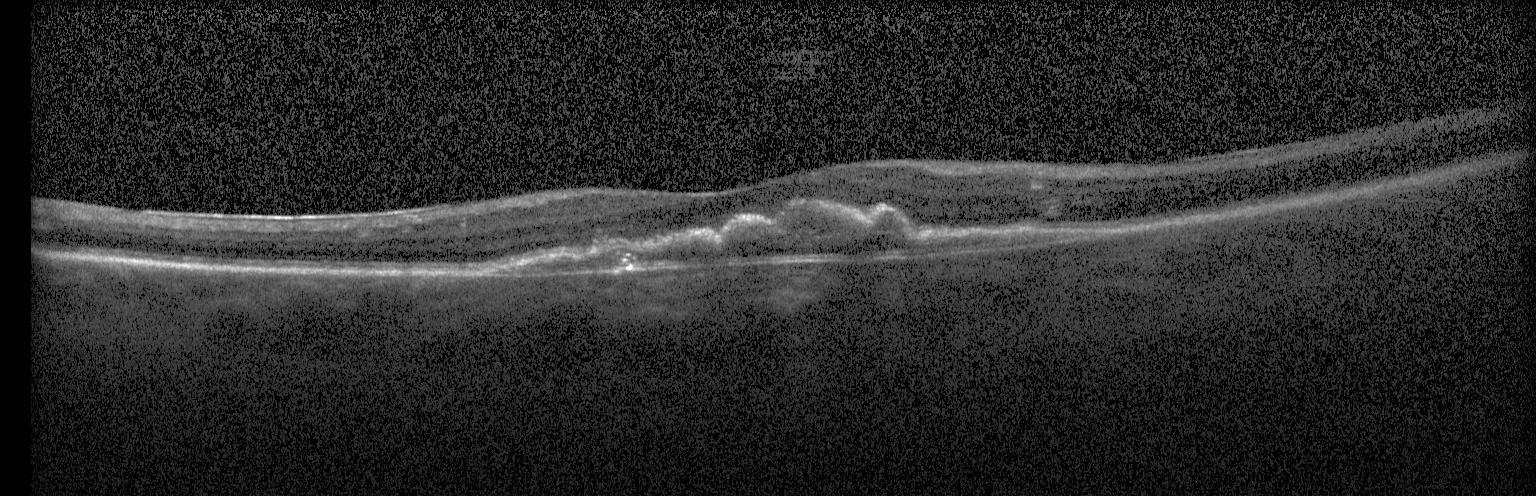 Retinal OCT cross-section, SD-OCT, centered on the fovea, instrument: Heidelberg Spectralis.
Impression: a choroidal neovascular membrane.